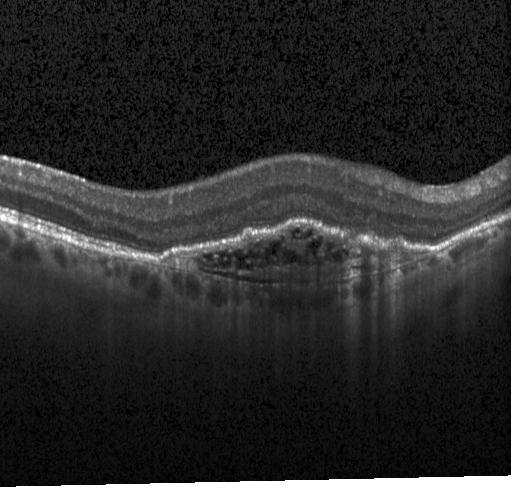

Retinal OCT cross-section
Diagnosis: a choroidal neovascular membrane.